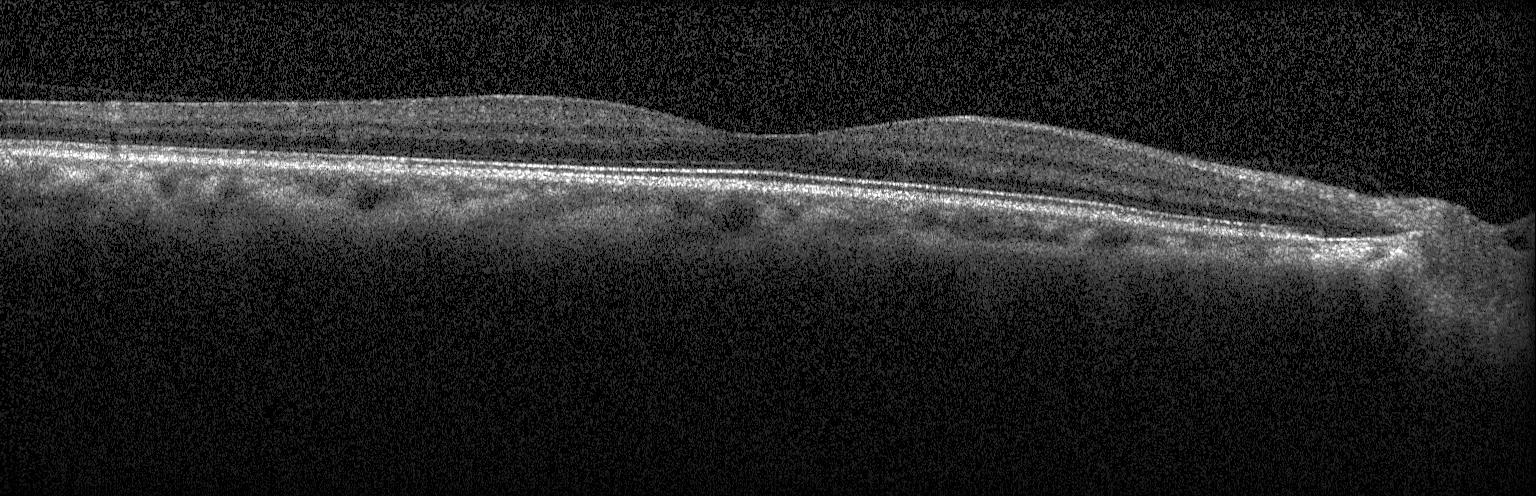

Optical coherence tomography scan. Diagnosis: no choroidal neovascularization, no diabetic macular edema, and no drusen.